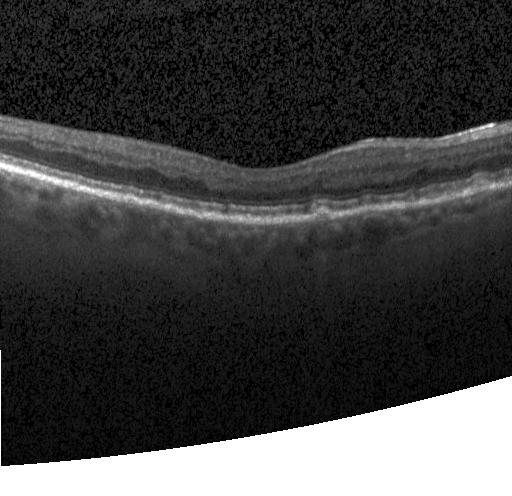
OCT B-scan showing drusen.